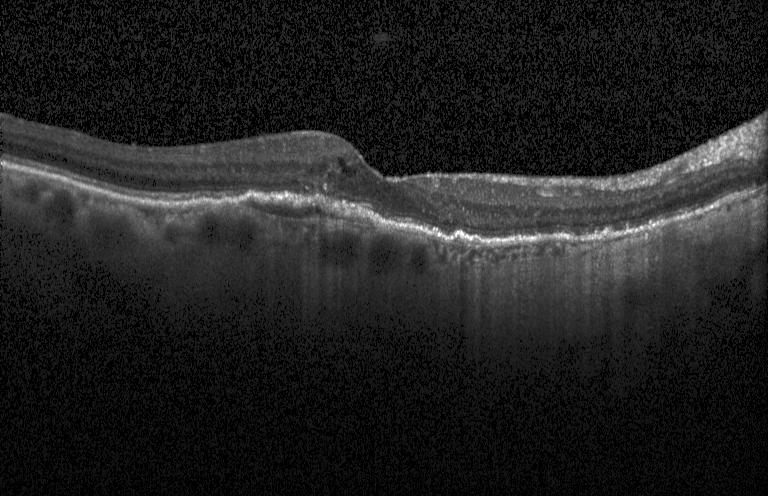

Spectral-domain OCT; macular scan; optical coherence tomography B-scan; Heidelberg Spectralis.
Dx: a choroidal neovascular membrane.